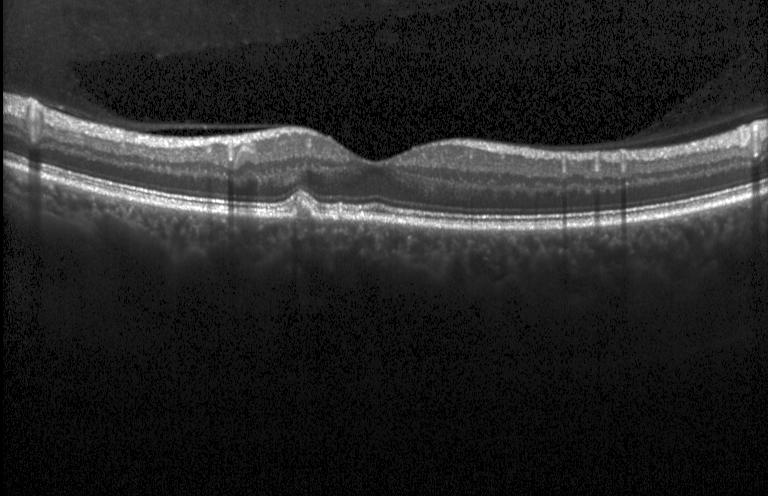 OCT line scan; macular scan; Heidelberg Spectralis OCT system. Impression: multiple drusen.